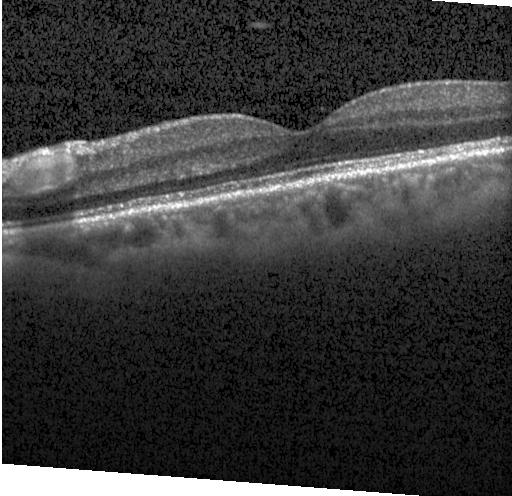
Macular OCT demonstrating no evidence of choroidal neovascularization, diabetic macular edema, or drusen.